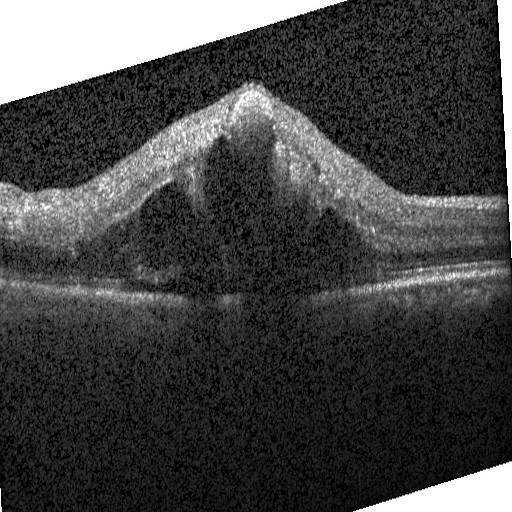 Instrument: Heidelberg Spectralis · spectral-domain optical coherence tomography · fovea-centered · optical coherence tomography scan.
Diabetic macular edema (DME).